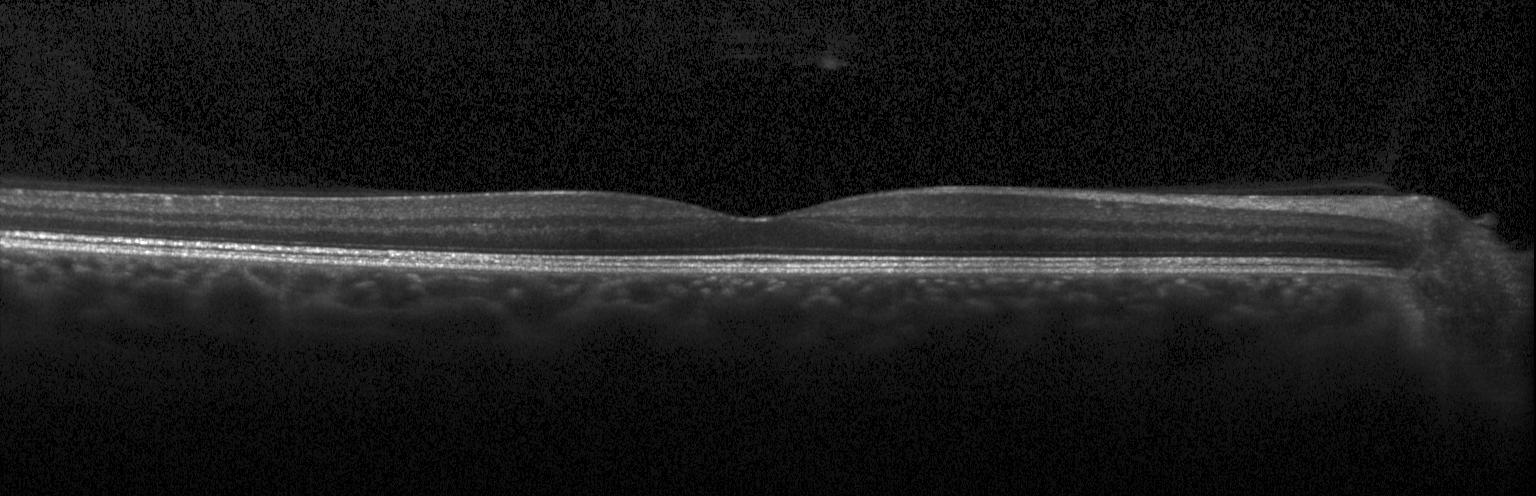 Finding: neither CNV, DME, nor drusen.